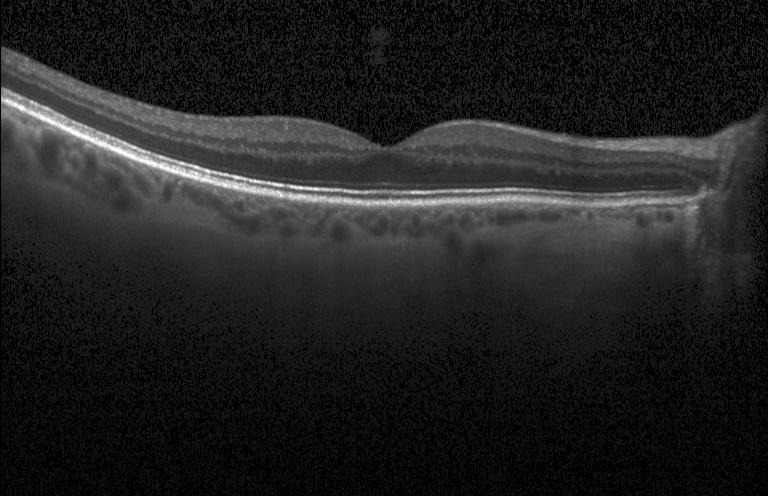

OCT B-scan showing no choroidal neovascularization, no diabetic macular edema, and no drusen.